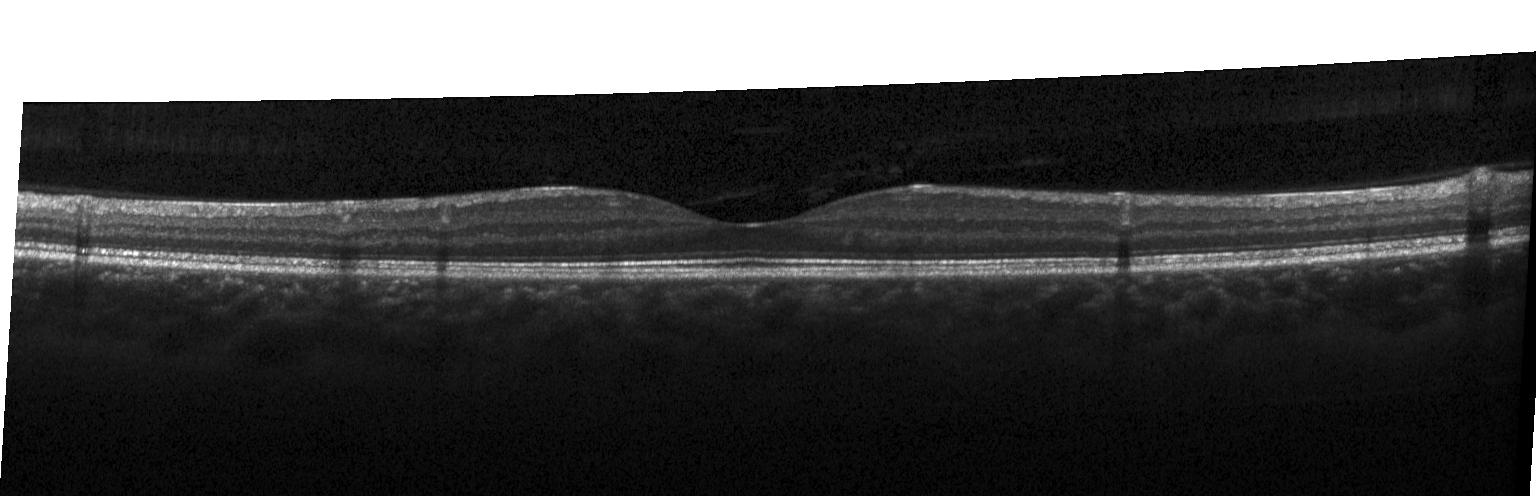
OCT B-scan showing no choroidal neovascularization, diabetic macular edema, or drusen.